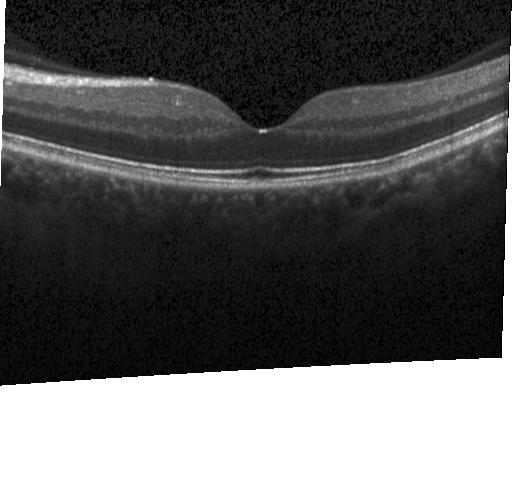

Optical coherence tomography scan · spectral-domain optical coherence tomography. Finding: no choroidal neovascularization, diabetic macular edema, or drusen.